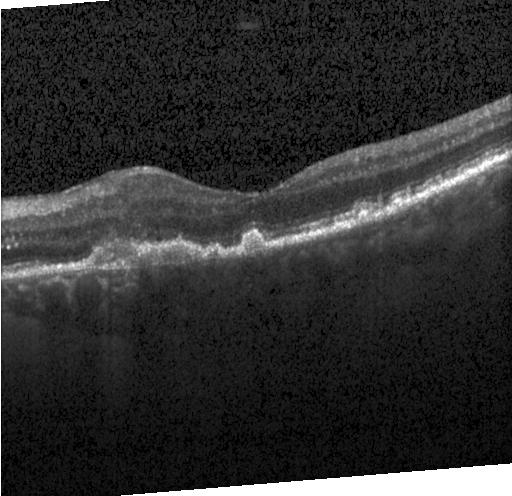
SD-OCT, retinal OCT B-scan. Impression: choroidal neovascularization.